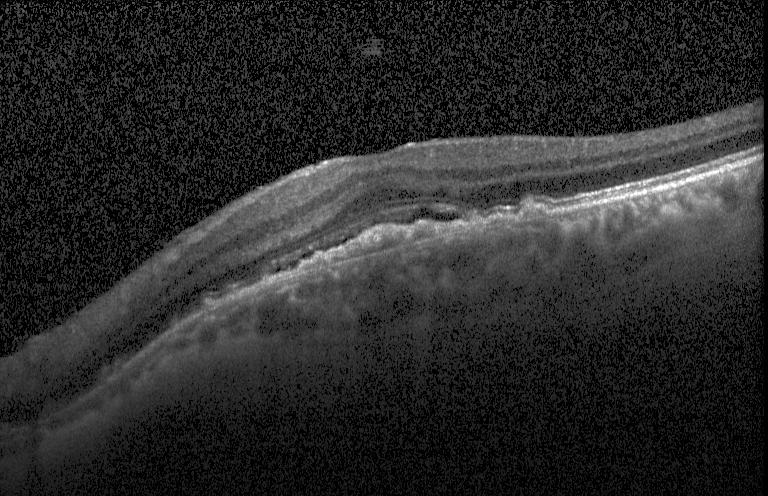

Impression: a choroidal neovascular membrane.